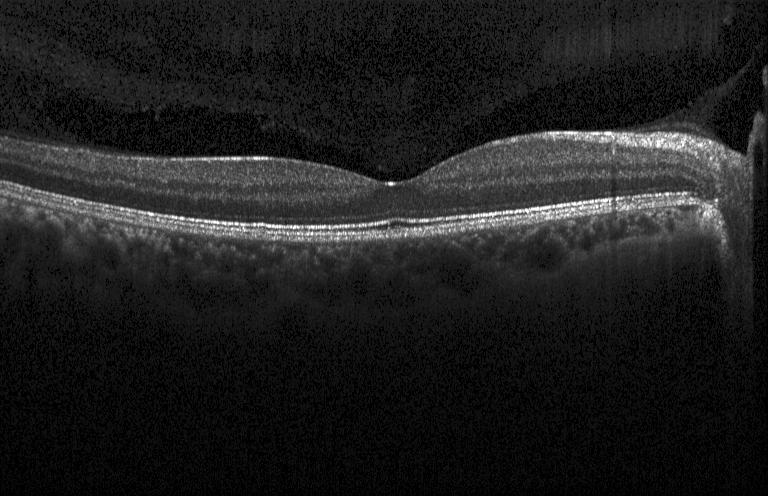 Optical coherence tomography scan. Impression: no CNV, DME, or drusen.